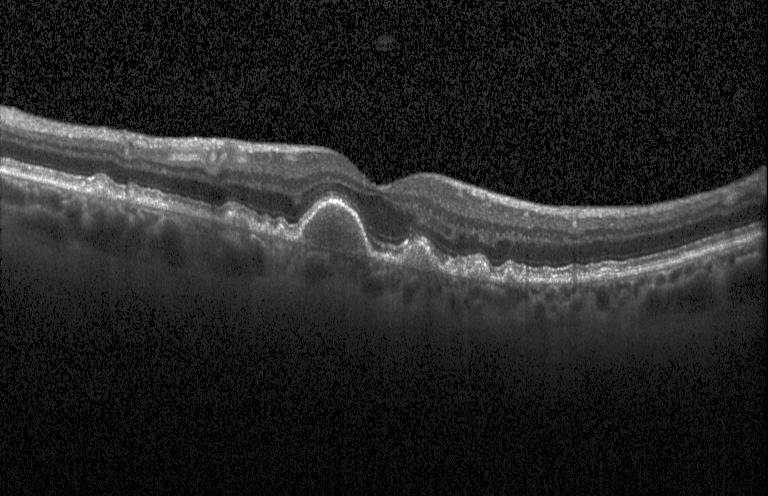

OCT finding: multiple drusen.